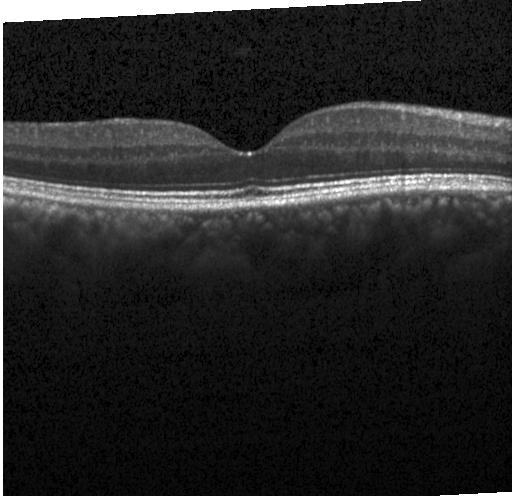

Optical coherence tomography B-scan — Diagnosis: no choroidal neovascularization, diabetic macular edema, or drusen.